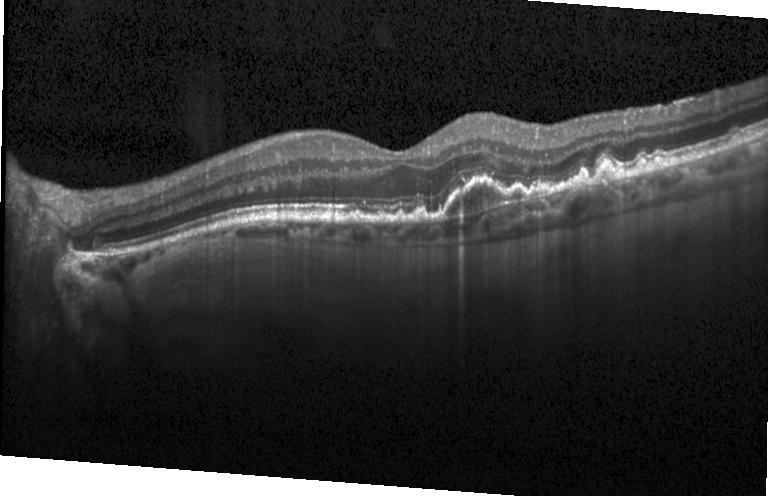
The scan shows a choroidal neovascular membrane.